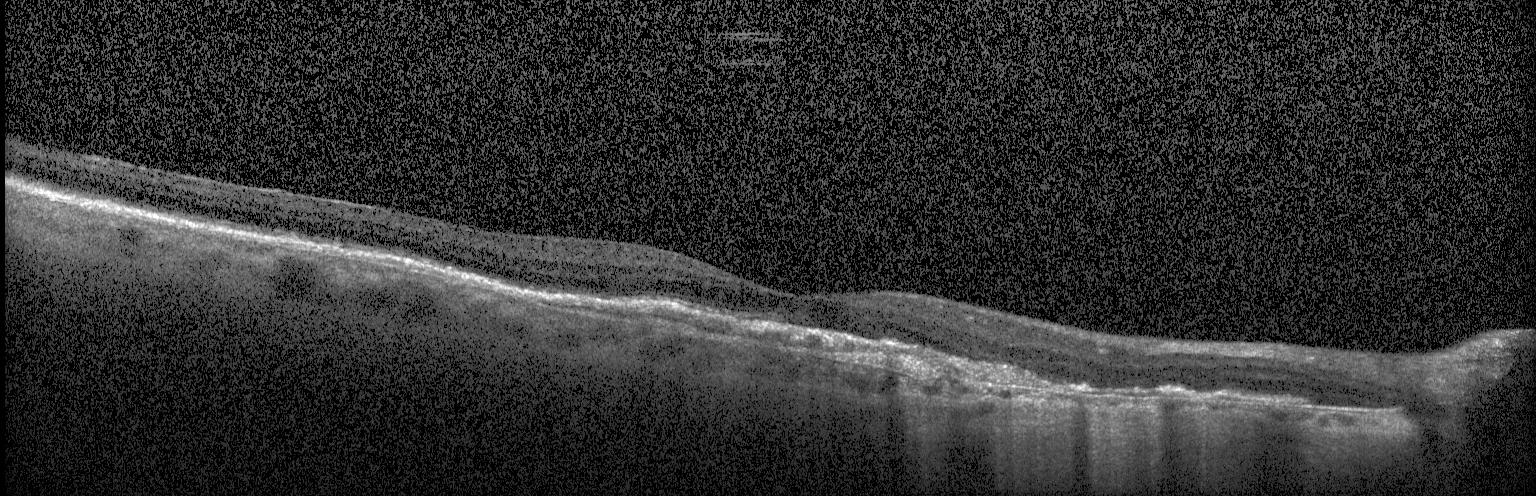 Dx: a choroidal neovascular membrane.